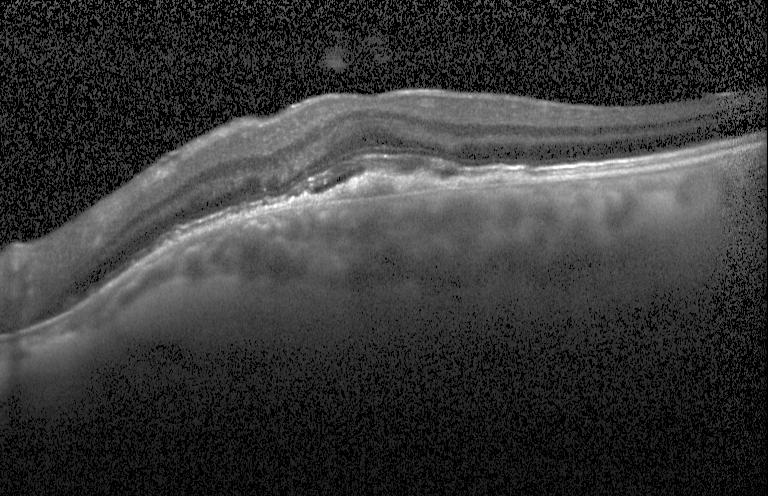

Acquired on a Heidelberg Spectralis, spectral-domain OCT, OCT line scan, through the macula. Impression: CNV.